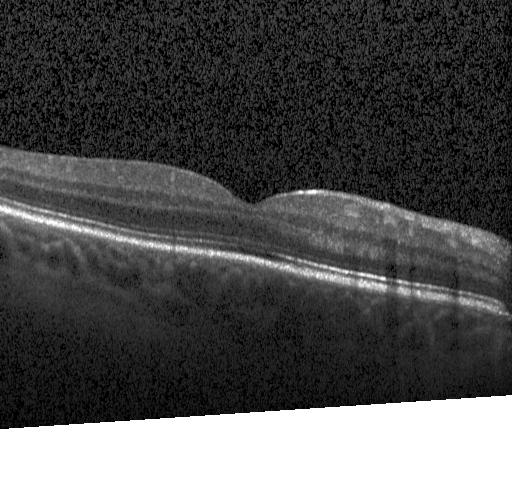

Centered on the fovea · retinal OCT B-scan · Heidelberg Spectralis OCT system · spectral-domain optical coherence tomography.
OCT finding: no CNV, DME, or drusen.